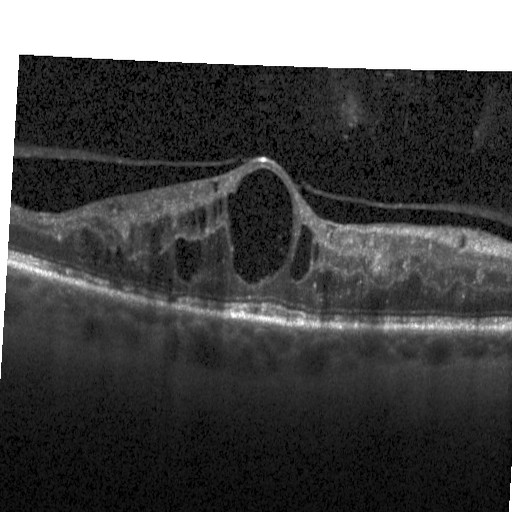

Impression: diabetic macular edema.